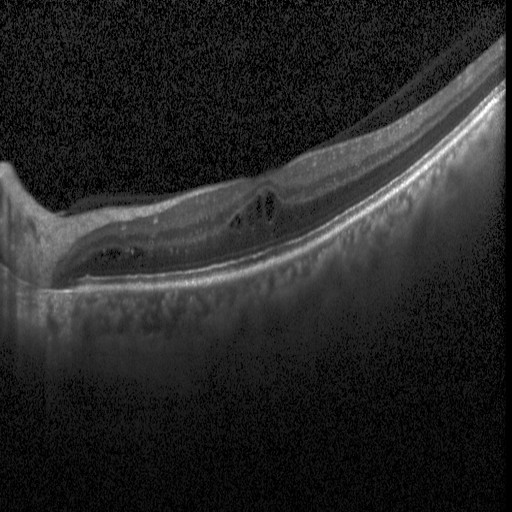

Retinal OCT B-scan
Diabetic macular edema.